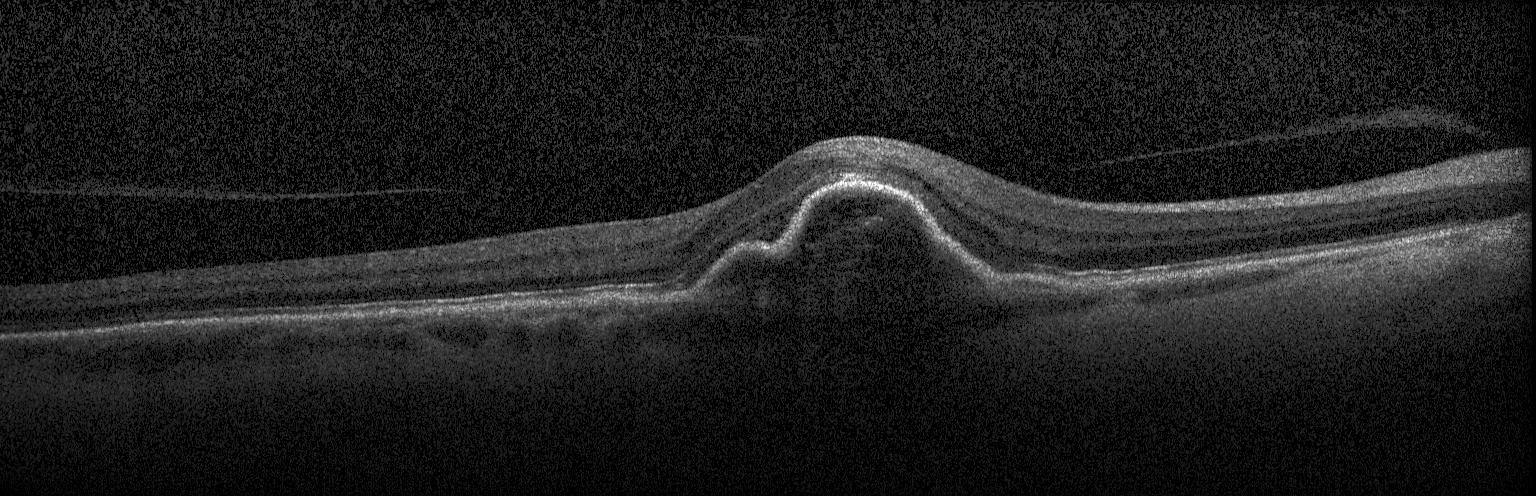

SD-OCT, OCT B-scan, macular scan. Dx: choroidal neovascularization.